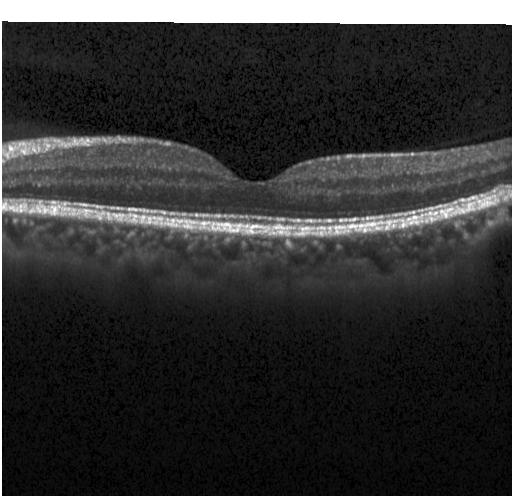 Optical coherence tomography B-scan; horizontal scan through the fovea; Heidelberg Spectralis OCT system; spectral-domain OCT.
Diagnosis: neither CNV, DME, nor drusen.